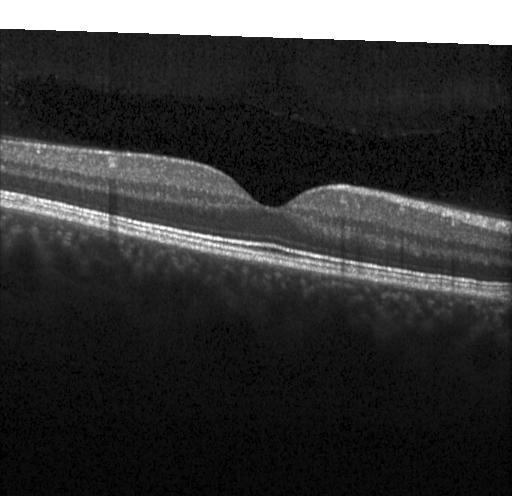
OCT B-scan showing no CNV, DME, or drusen.